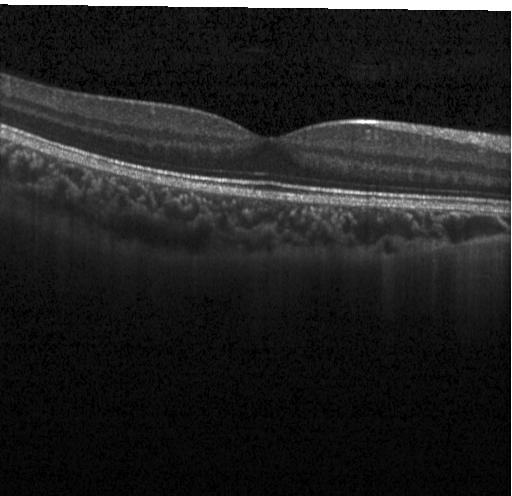

OCT finding: no CNV, DME, or drusen.